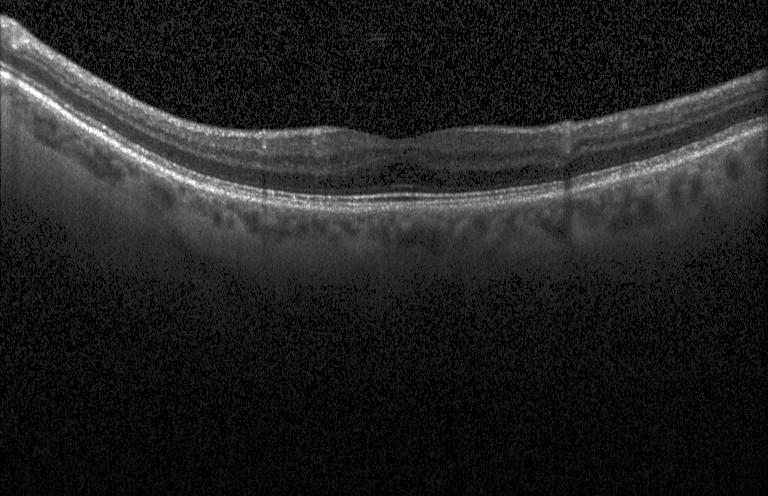

OCT finding: no choroidal neovascularization, no diabetic macular edema, and no drusen.